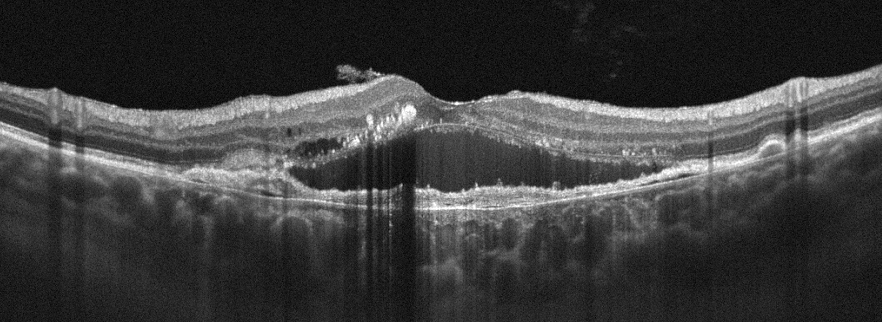
OD · OCT B-scan. Finding: AMD.